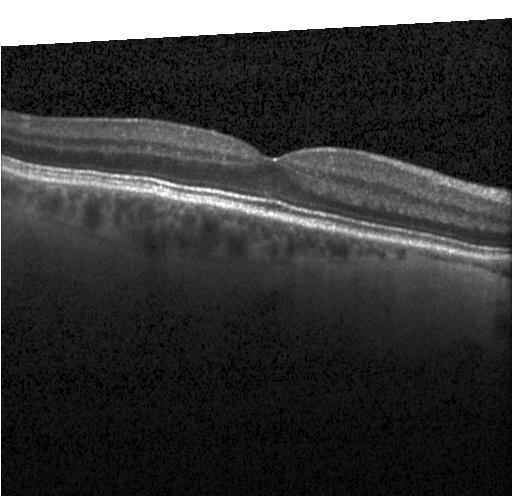 Optical coherence tomography scan; acquired on a Heidelberg Spectralis — OCT finding: no choroidal neovascularization, diabetic macular edema, or drusen.